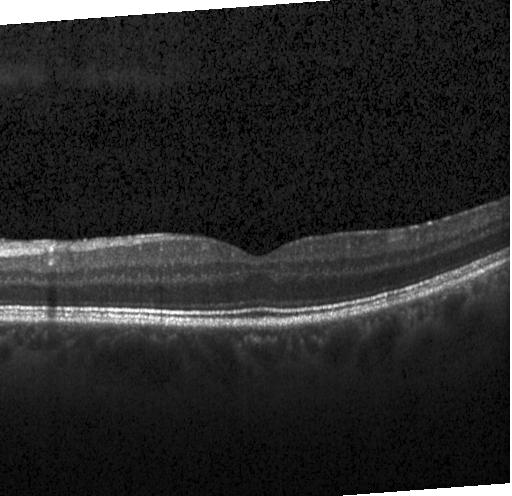

Retinal OCT B-scan. Fovea-centered. Spectral-domain optical coherence tomography.
Dx: neither choroidal neovascularization, diabetic macular edema, nor drusen.